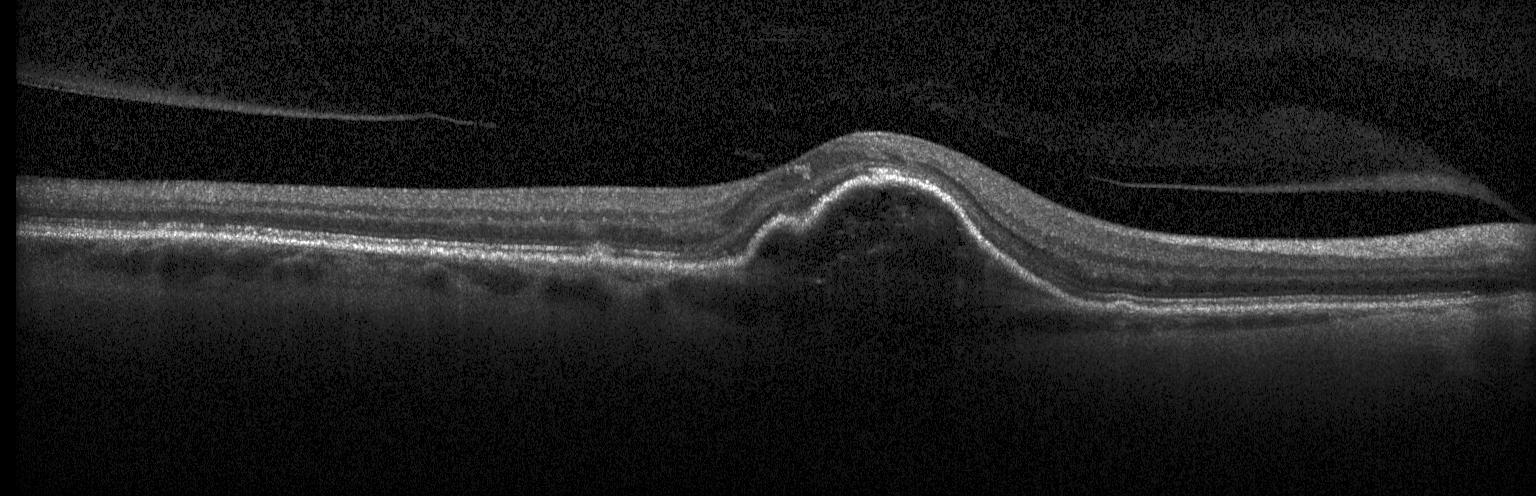
OCT B-scan; fovea-centered.
The scan shows a choroidal neovascular membrane.